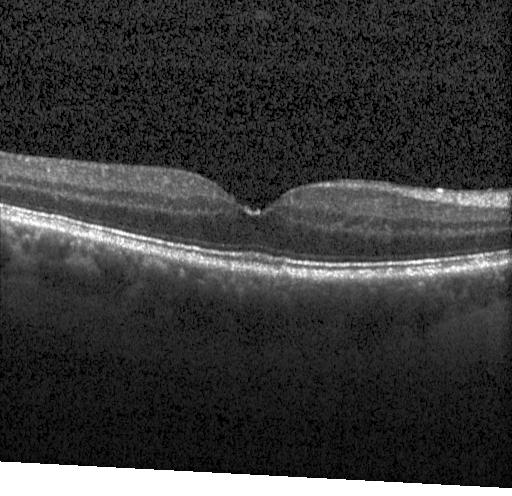

OCT B-scan showing multiple drusen.